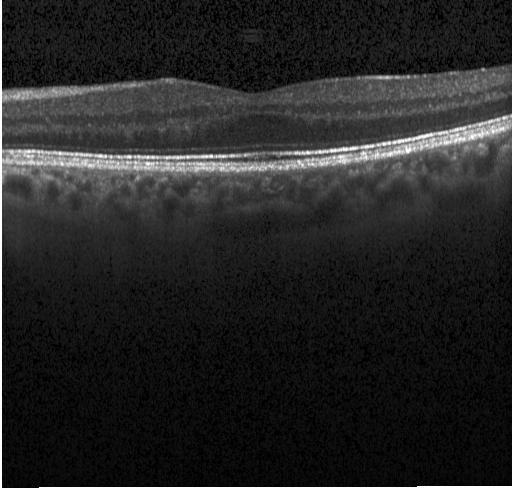
Dx: no choroidal neovascularization, no diabetic macular edema, and no drusen.